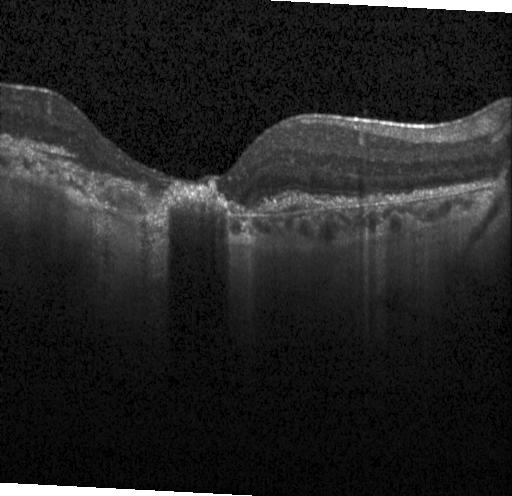

Spectral-domain OCT · horizontal scan through the fovea · retinal OCT cross-section — Assessment: a choroidal neovascular membrane.